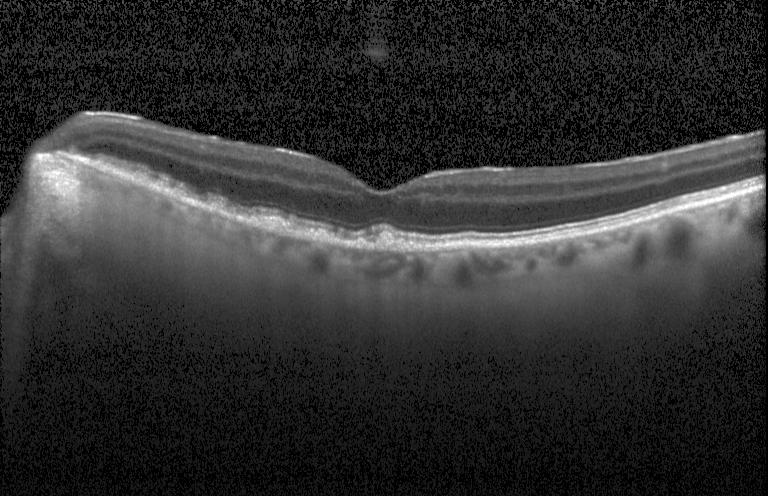
Retinal OCT cross-section showing sub-RPE drusenoid deposits.